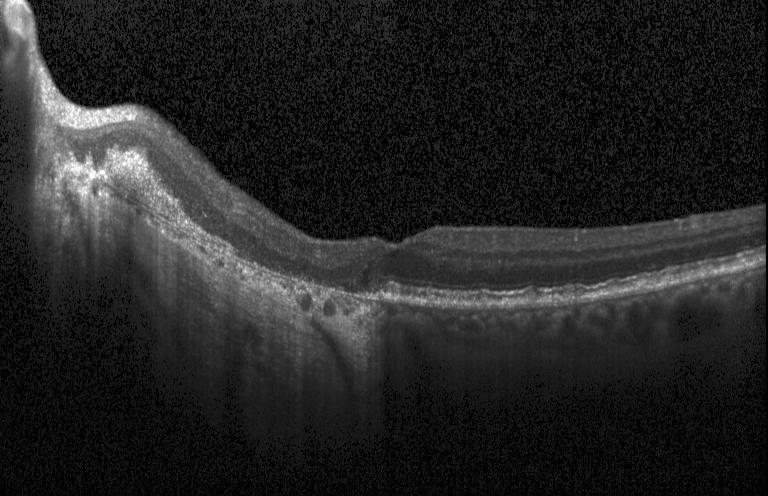
OCT finding: choroidal neovascularization.